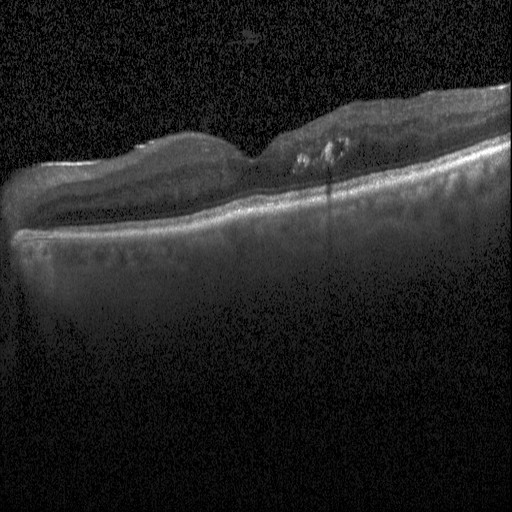 Retinal OCT cross-section showing diabetic macular edema.